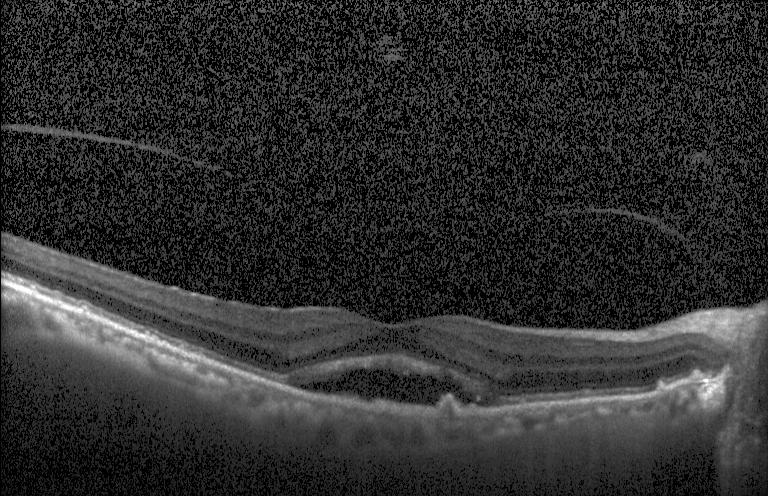

This B-scan demonstrates choroidal neovascularization.